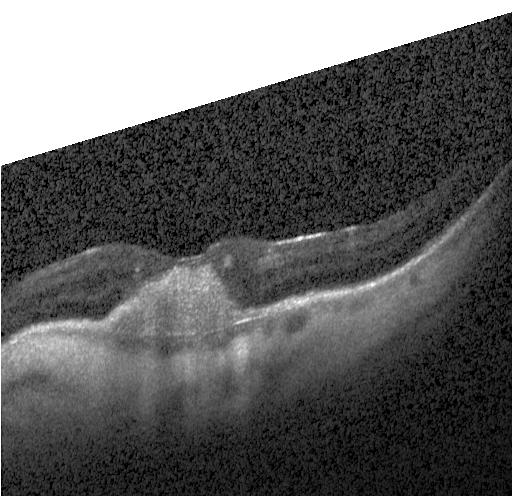

Acquired on a Heidelberg Spectralis · retinal OCT B-scan — Diagnosis: a choroidal neovascular membrane.